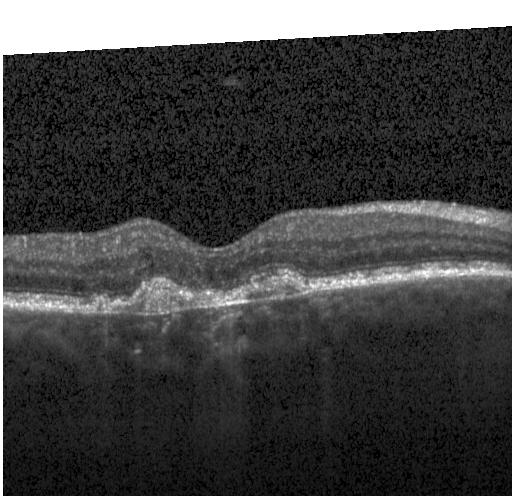 OCT line scan · horizontal scan through the fovea — Dx: CNV.